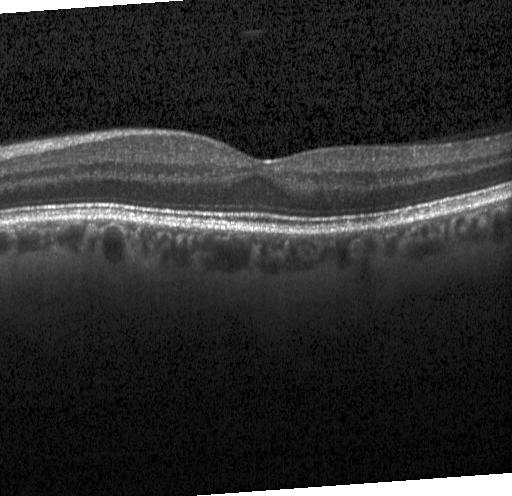 Spectral-domain OCT; Heidelberg Spectralis OCT system; retinal OCT cross-section; through the macula
This B-scan demonstrates no choroidal neovascularization, diabetic macular edema, or drusen.